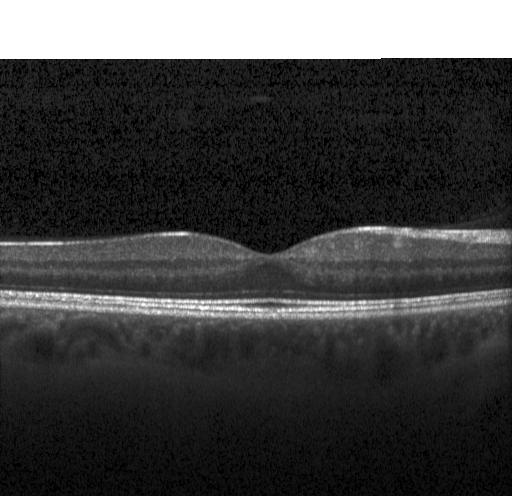

Optical coherence tomography B-scan, macular scan, spectral-domain optical coherence tomography, Heidelberg Spectralis
Diagnosis: no choroidal neovascularization, no diabetic macular edema, and no drusen.